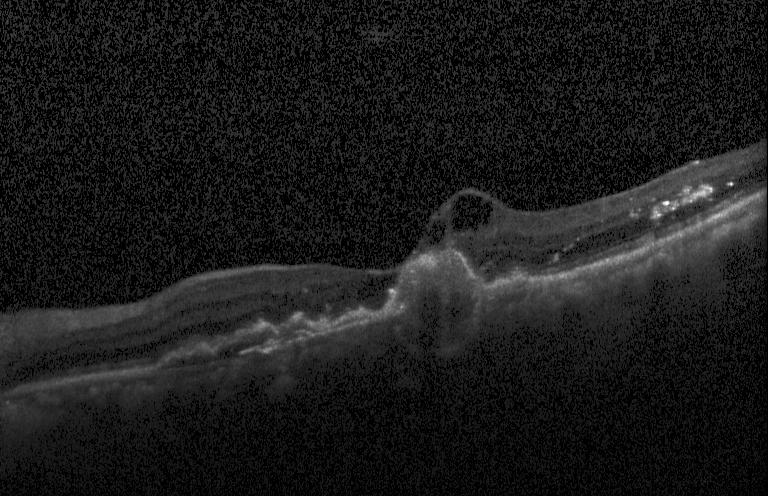
Retinal OCT cross-section showing choroidal neovascularization (CNV).